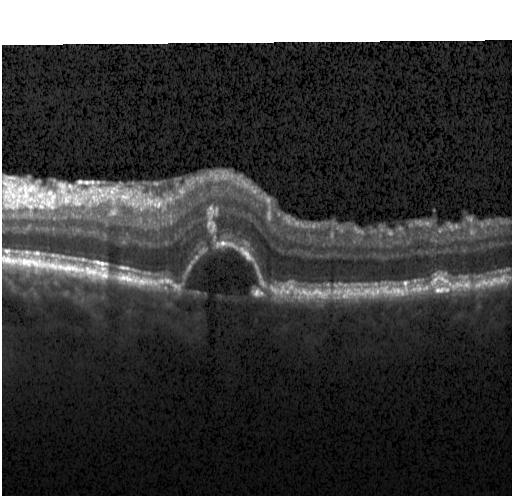 The scan shows choroidal neovascularization.